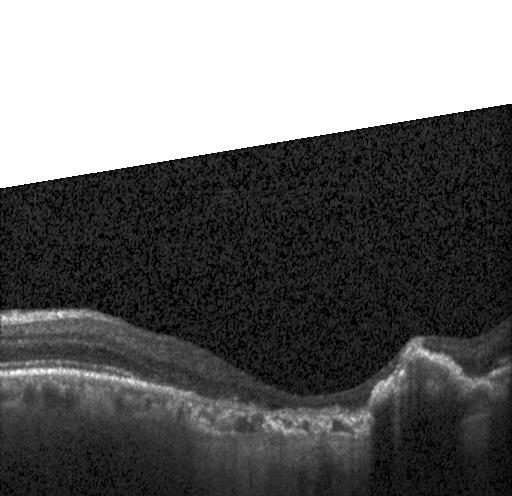

Heidelberg Spectralis OCT system; OCT B-scan; horizontal scan through the fovea — Impression: a choroidal neovascular membrane.